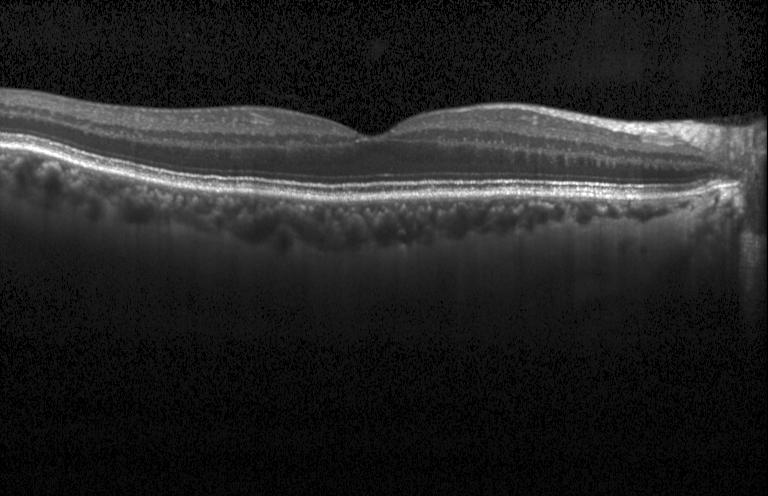 Spectral-domain optical coherence tomography; OCT line scan. Diagnosis: no choroidal neovascularization, no diabetic macular edema, and no drusen.